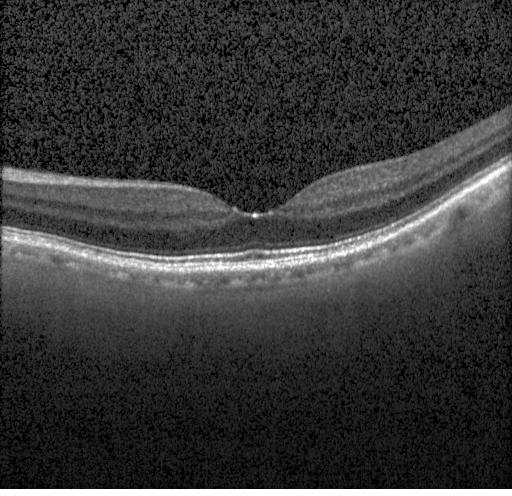
Retinal OCT cross-section, spectral-domain OCT — Diagnosis: no choroidal neovascularization, no diabetic macular edema, and no drusen.